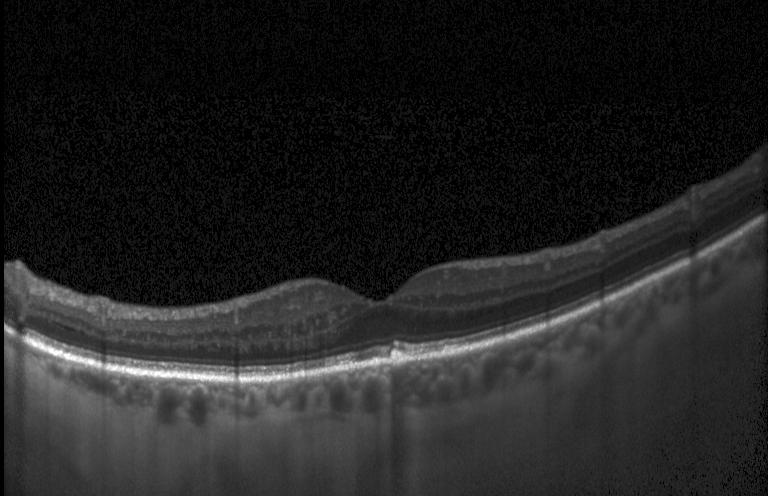

Diagnosis: sub-RPE drusenoid deposits.